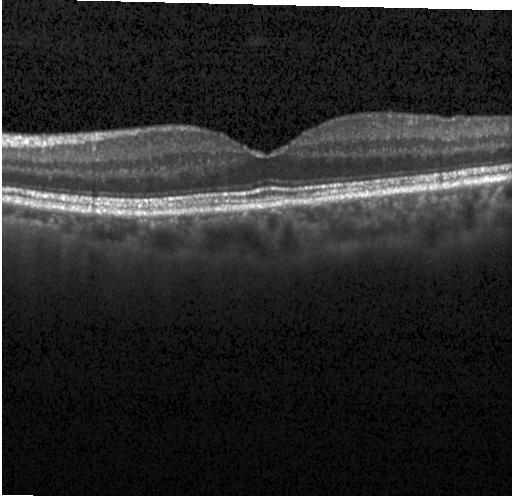

Optical coherence tomography scan, fovea-centered
Impression: neither CNV, DME, nor drusen.